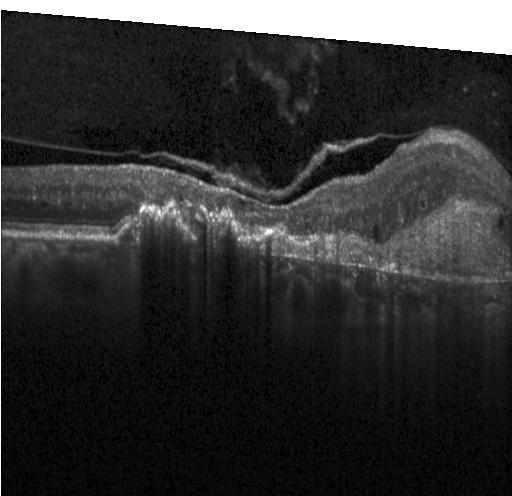
Macular OCT: a choroidal neovascular membrane.